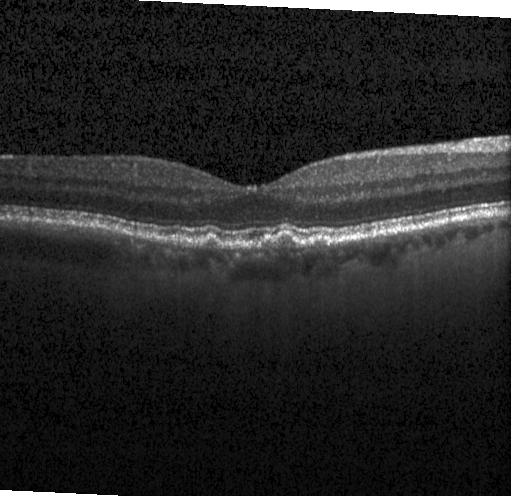
Finding: sub-RPE drusenoid deposits.